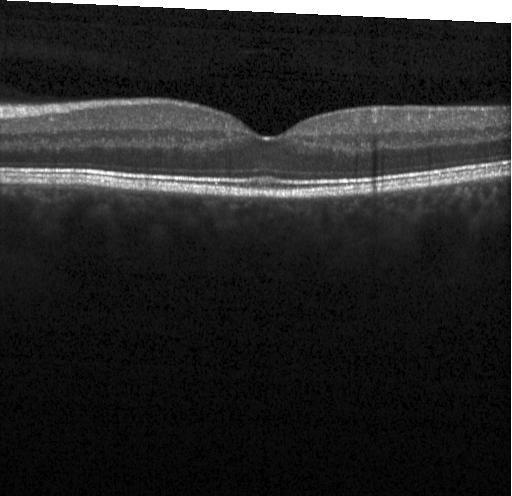 This B-scan demonstrates neither choroidal neovascularization, diabetic macular edema, nor drusen.